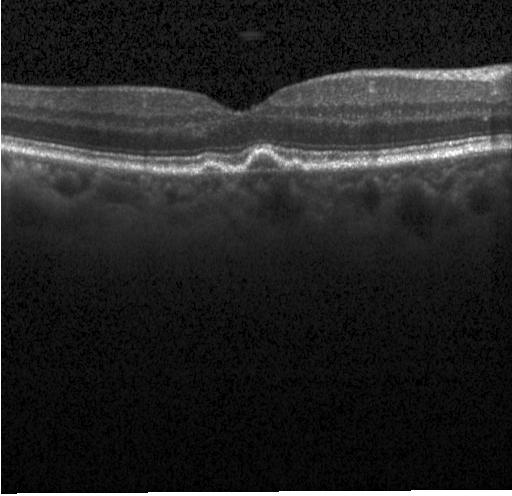
Impression: sub-RPE drusenoid deposits.